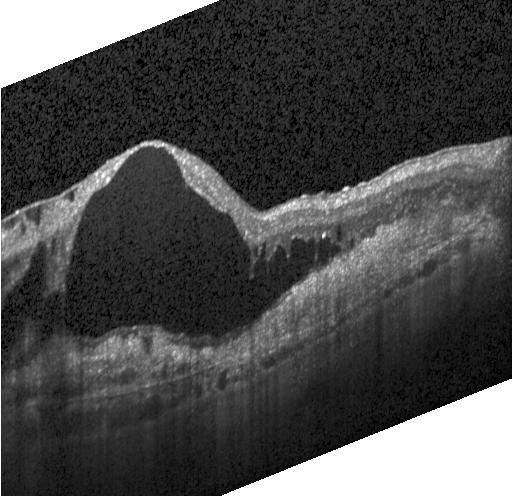
Spectral-domain OCT. Heidelberg Spectralis. Optical coherence tomography B-scan — The scan shows choroidal neovascularization.